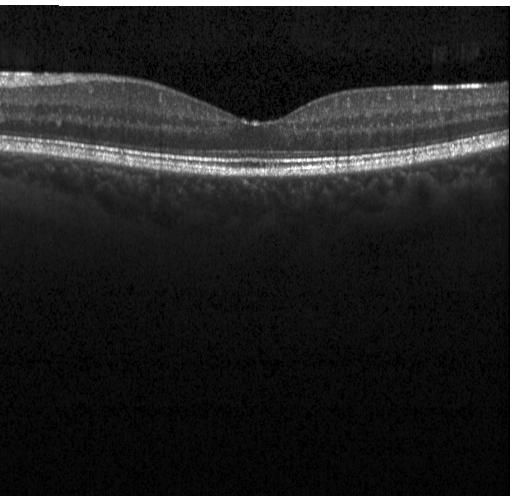 Spectral-domain OCT, optical coherence tomography scan, acquired on a Heidelberg Spectralis, horizontal scan through the fovea. Diagnosis: neither CNV, DME, nor drusen.